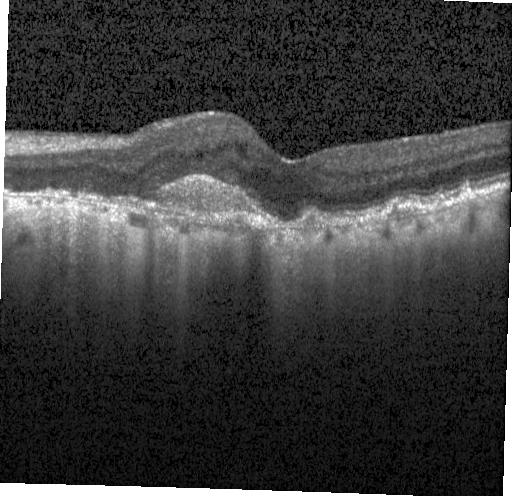
Horizontal scan through the fovea; Heidelberg Spectralis; OCT line scan.
Dx: a choroidal neovascular membrane.